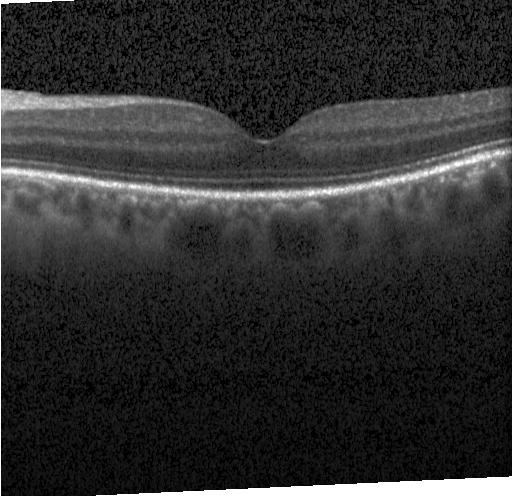 OCT B-scan showing no choroidal neovascularization, no diabetic macular edema, and no drusen.